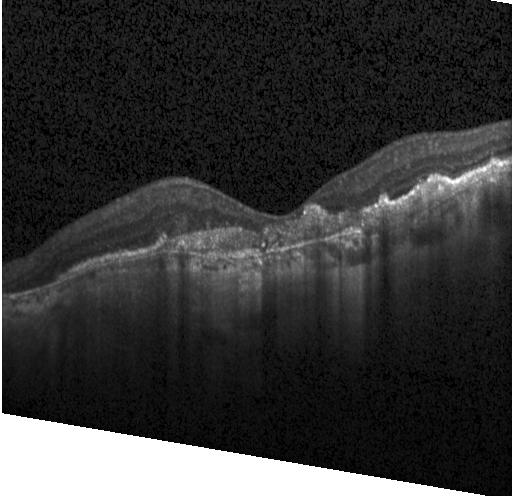
Retinal OCT cross-section · macular scan.
Diagnosis: choroidal neovascularization.